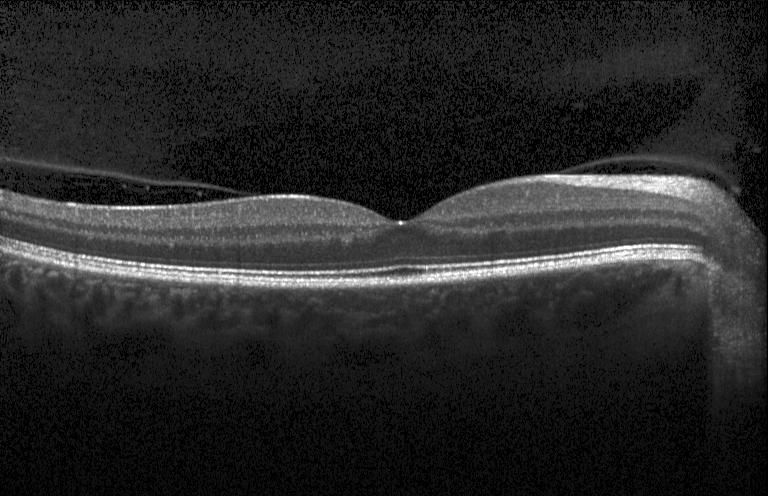
OCT B-scan, spectral-domain optical coherence tomography.
Impression: no CNV, DME, or drusen.